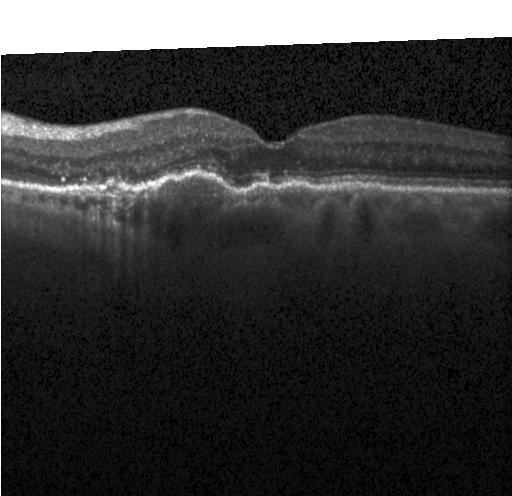
Macular scan, optical coherence tomography B-scan, SD-OCT — Choroidal neovascularization (CNV).